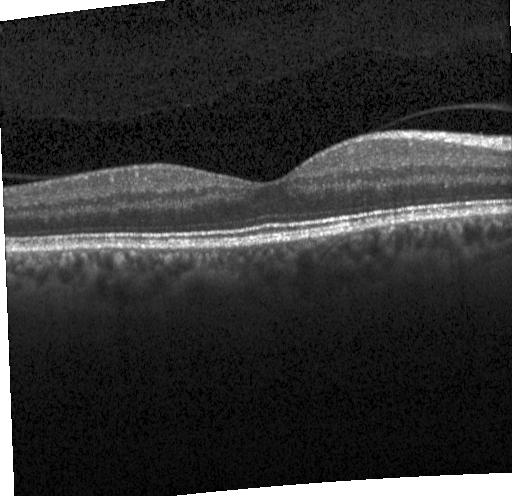
Optical coherence tomography B-scan · Heidelberg Spectralis OCT system · macular scan.
Impression: no CNV, no DME, and no drusen.